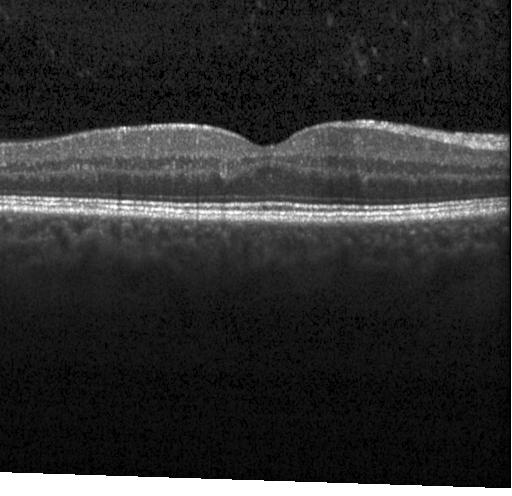
This B-scan demonstrates neither CNV, DME, nor drusen.